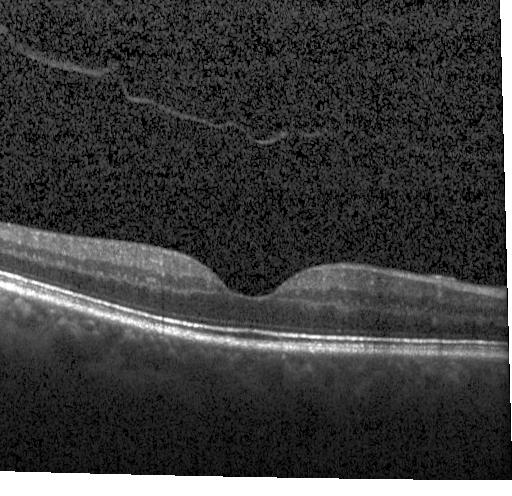
SD-OCT; through the macula; retinal OCT cross-section
OCT finding: no evidence of choroidal neovascularization, diabetic macular edema, or drusen.